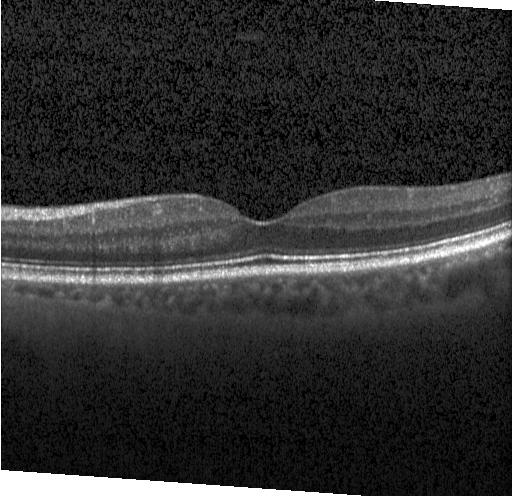

Diagnosis: no choroidal neovascularization, diabetic macular edema, or drusen.